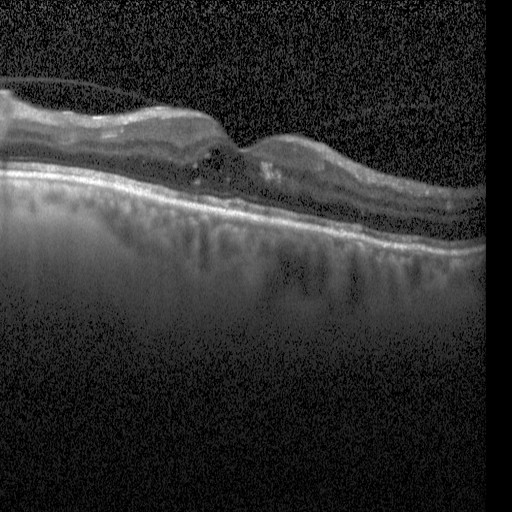 SD-OCT · OCT B-scan · Heidelberg Spectralis OCT system — Assessment: DME.